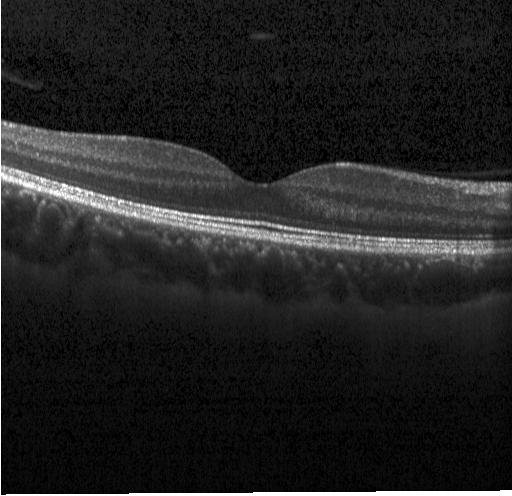
Retinal OCT B-scan
Macular OCT: neither choroidal neovascularization, diabetic macular edema, nor drusen.